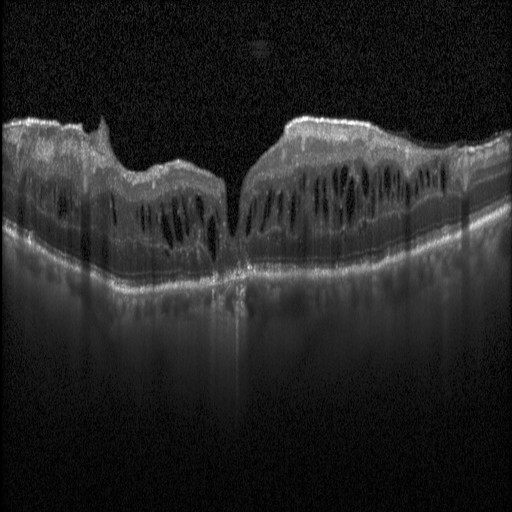 Macular scan. Spectral-domain OCT. OCT B-scan — Finding: diabetic macular edema.